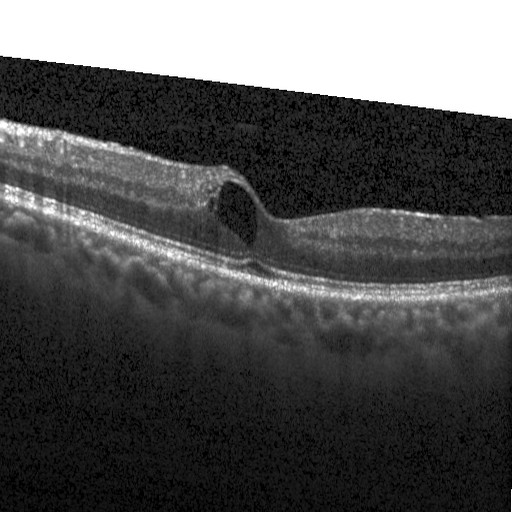 OCT B-scan. Heidelberg Spectralis OCT system.
The scan shows DME.